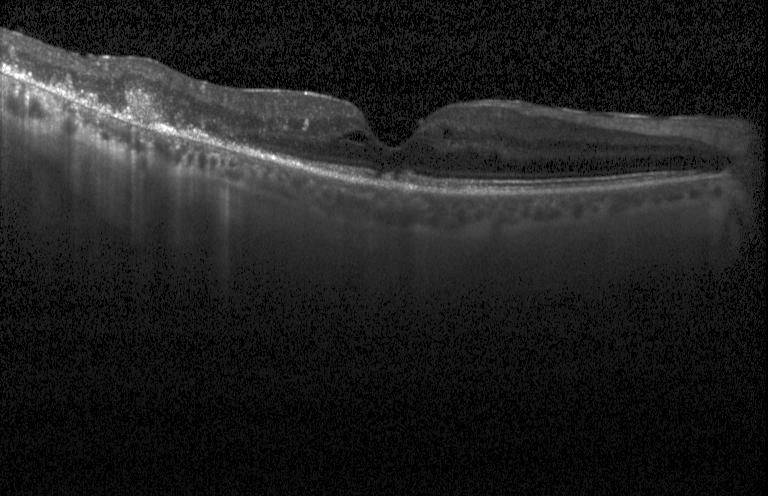 Retinal OCT cross-section.
Impression: a choroidal neovascular membrane.